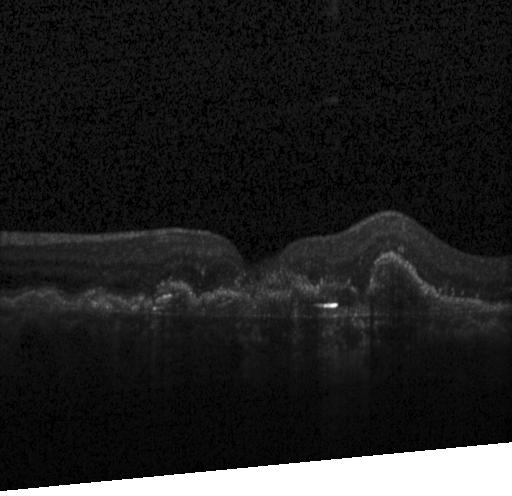
Optical coherence tomography B-scan — Diagnosis: a choroidal neovascular membrane.